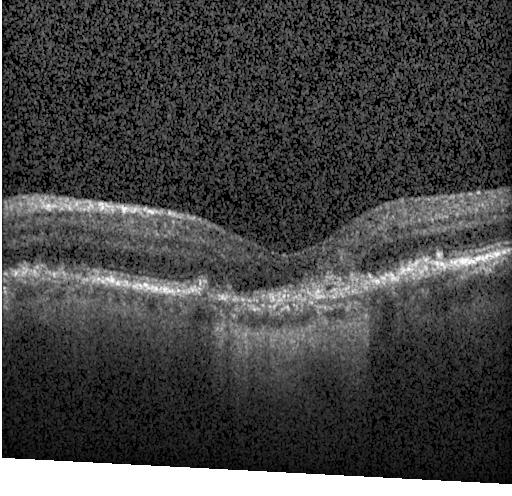
Optical coherence tomography B-scan. SD-OCT. Heidelberg Spectralis OCT system. Fovea-centered — Impression: a choroidal neovascular membrane.